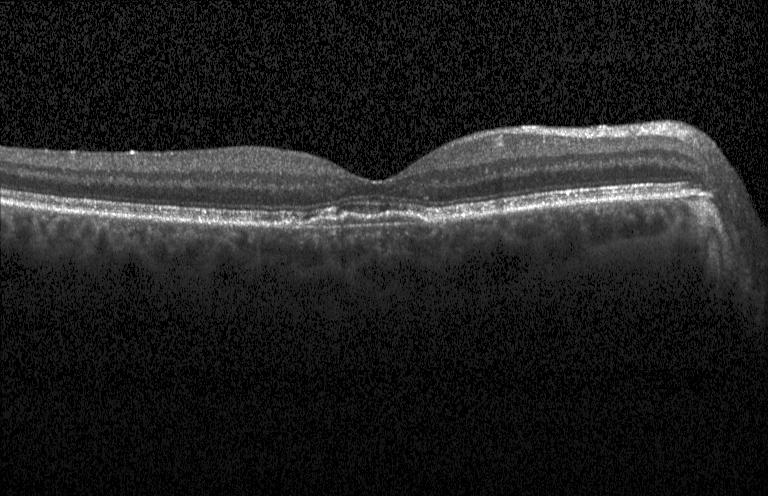
Spectral-domain OCT B-scan: CNV.